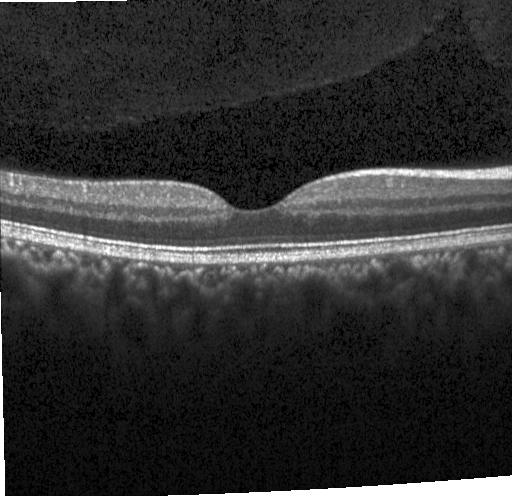 Spectral-domain OCT · through the macula · optical coherence tomography scan · Heidelberg Spectralis
Diagnosis: no choroidal neovascularization, diabetic macular edema, or drusen.